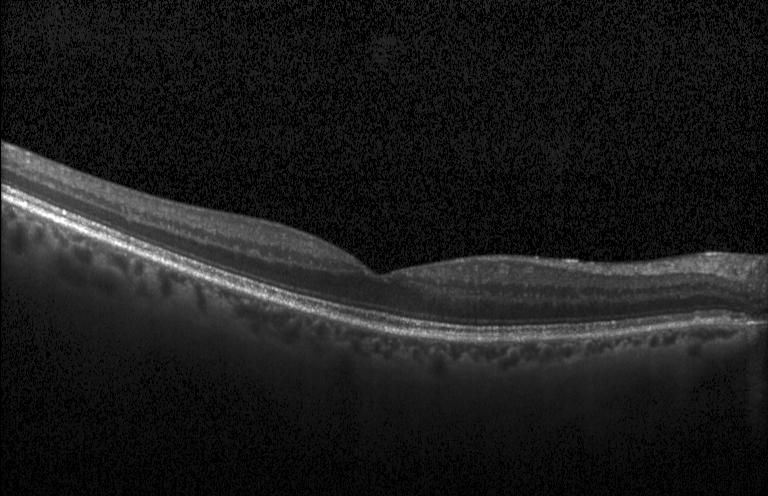 Instrument: Heidelberg Spectralis · macular scan · spectral-domain OCT · optical coherence tomography scan.
Diagnosis: no choroidal neovascularization, diabetic macular edema, or drusen.